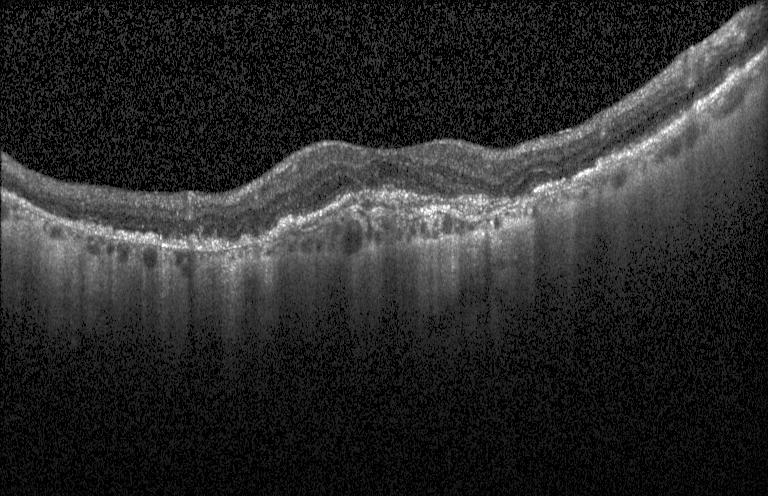 Optical coherence tomography scan; SD-OCT; Heidelberg Spectralis OCT system
Diagnosis: a choroidal neovascular membrane.